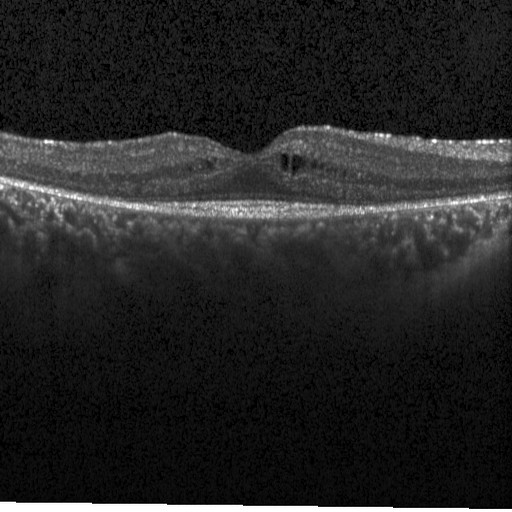 Retinal OCT B-scan — This B-scan demonstrates DME.